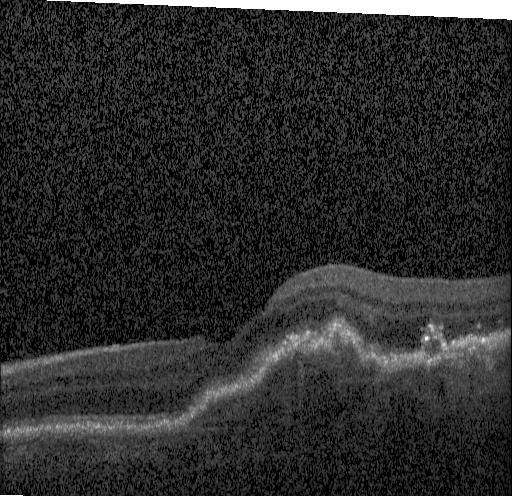
Spectral-domain optical coherence tomography; OCT B-scan
Assessment: a choroidal neovascular membrane.